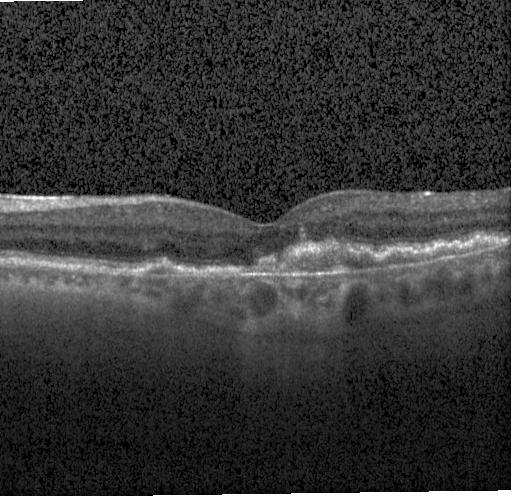
SD-OCT. OCT line scan. Heidelberg Spectralis. Horizontal scan through the fovea — Finding: choroidal neovascularization.